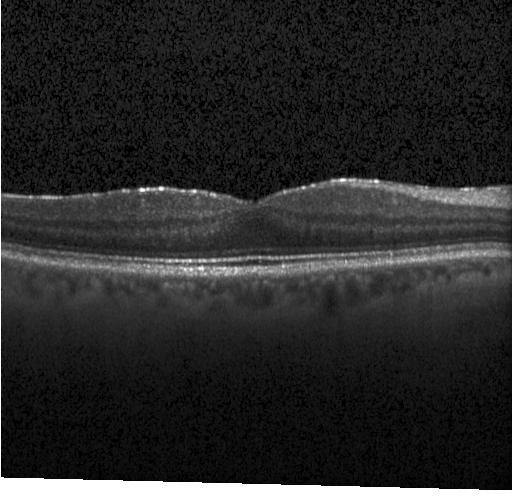
Optical coherence tomography B-scan
Finding: no evidence of choroidal neovascularization, diabetic macular edema, or drusen.